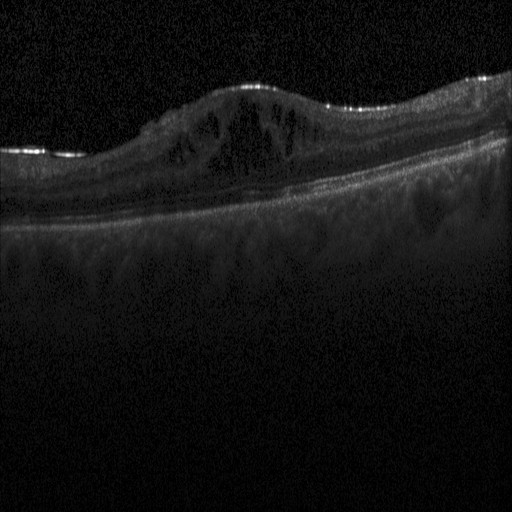

Retinal OCT cross-section; centered on the fovea
Impression: diabetic macular edema (DME).